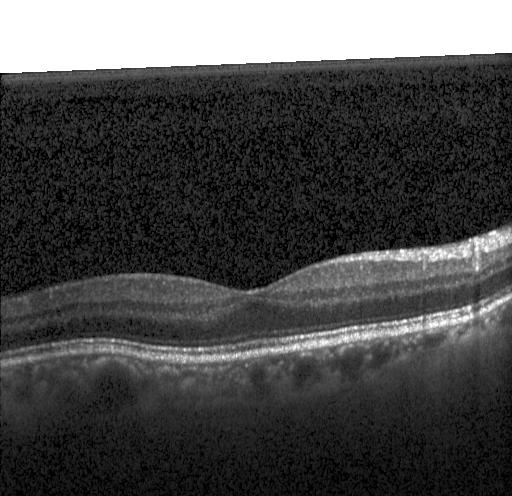

Diagnosis: neither choroidal neovascularization, diabetic macular edema, nor drusen.